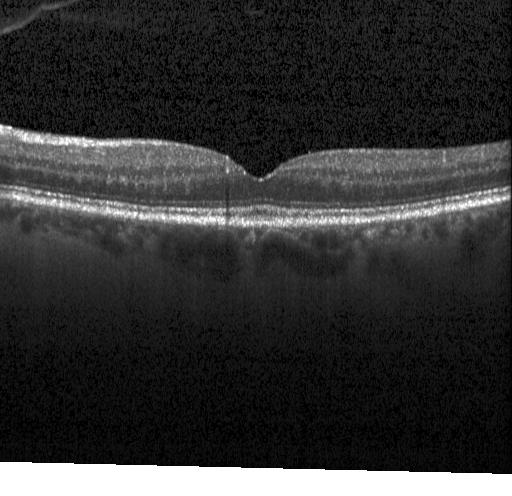
Macular OCT: no evidence of choroidal neovascularization, diabetic macular edema, or drusen.